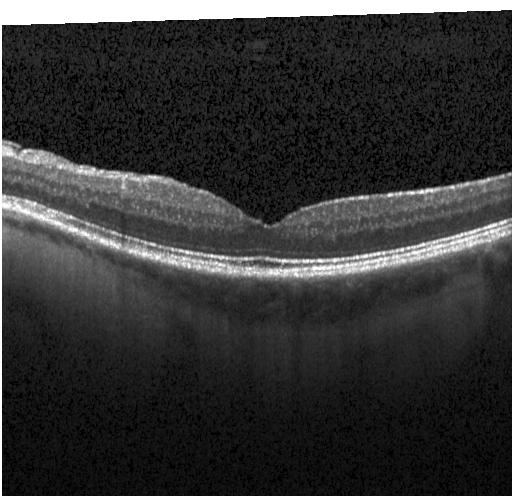
Assessment: no choroidal neovascularization, no diabetic macular edema, and no drusen.